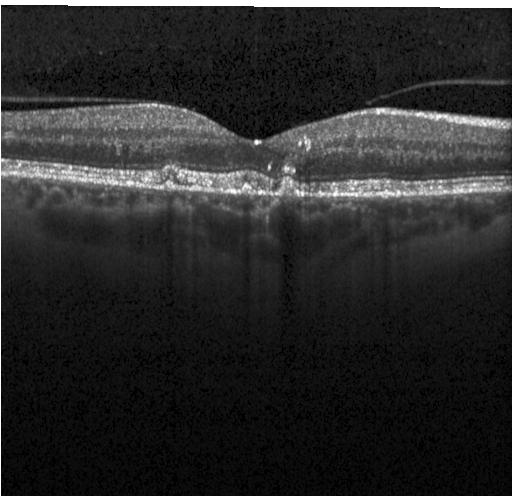
OCT B-scan showing drusen.